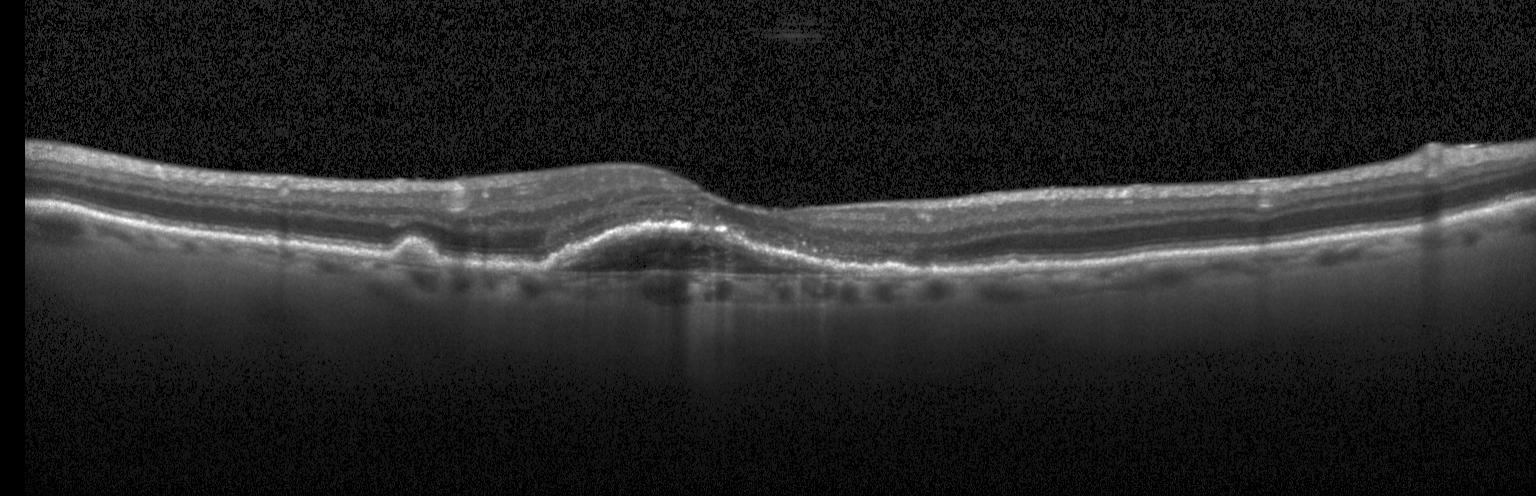
Impression: choroidal neovascularization.